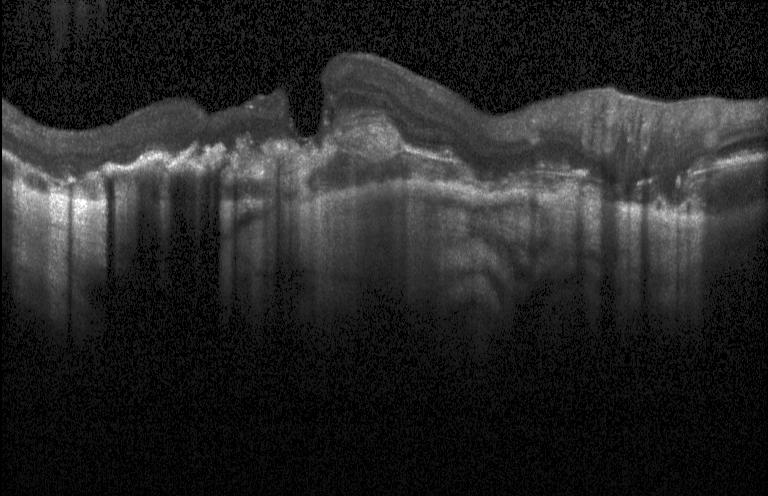
Retinal OCT cross-section, acquired on a Heidelberg Spectralis, spectral-domain optical coherence tomography, horizontal scan through the fovea.
The scan shows choroidal neovascularization (CNV).